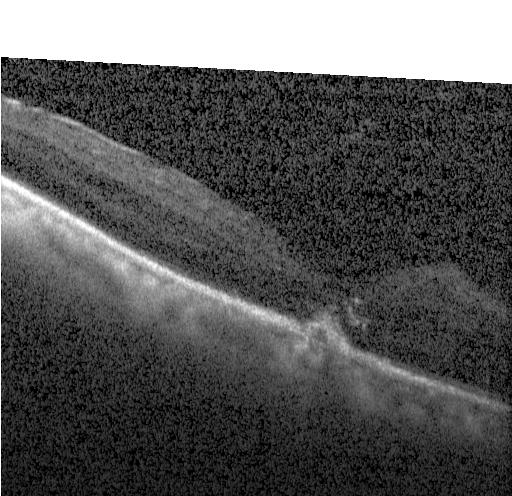 Spectral-domain optical coherence tomography; acquired on a Heidelberg Spectralis; centered on the fovea; OCT B-scan
Assessment: a choroidal neovascular membrane.